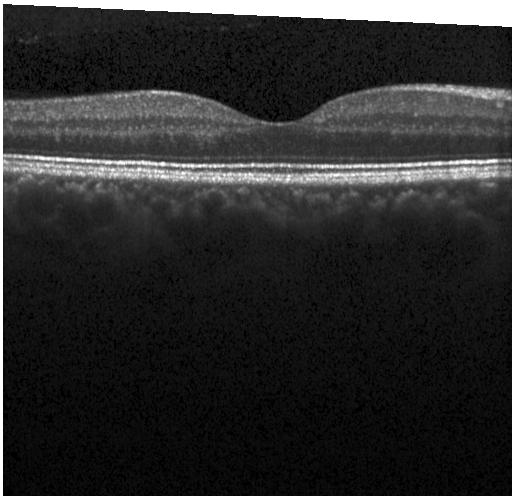

OCT B-scan.
Assessment: no CNV, no DME, and no drusen.